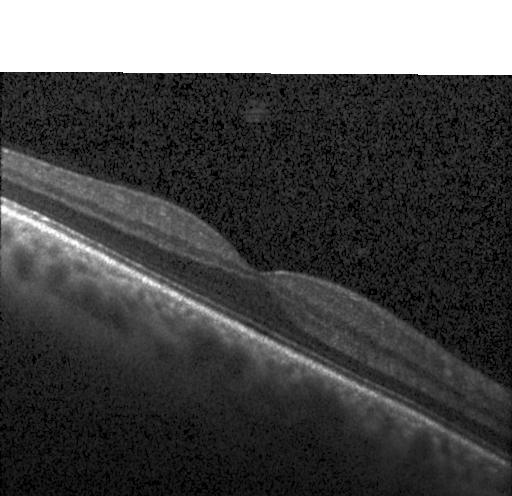
Neither choroidal neovascularization, diabetic macular edema, nor drusen.